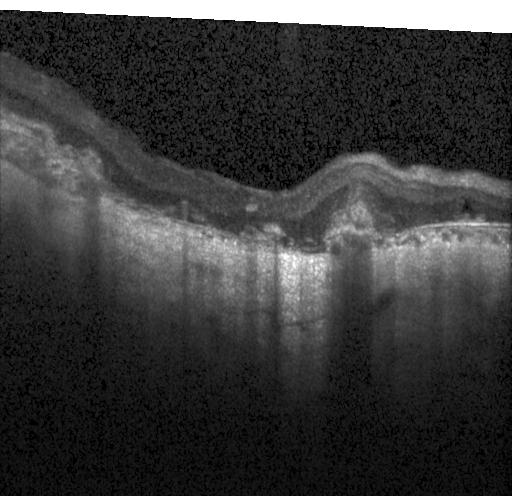

Through the macula, spectral-domain optical coherence tomography, Heidelberg Spectralis, OCT line scan — Macular OCT: a choroidal neovascular membrane.